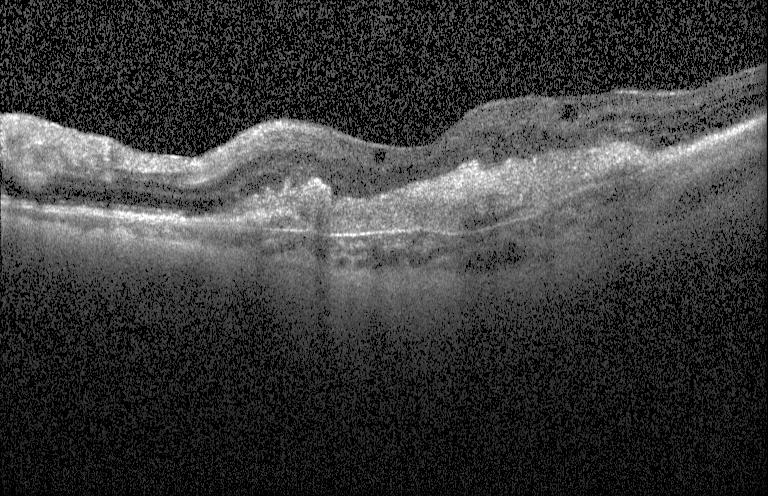
Through the macula · acquired on a Heidelberg Spectralis · SD-OCT · OCT line scan
Diagnosis: a choroidal neovascular membrane.